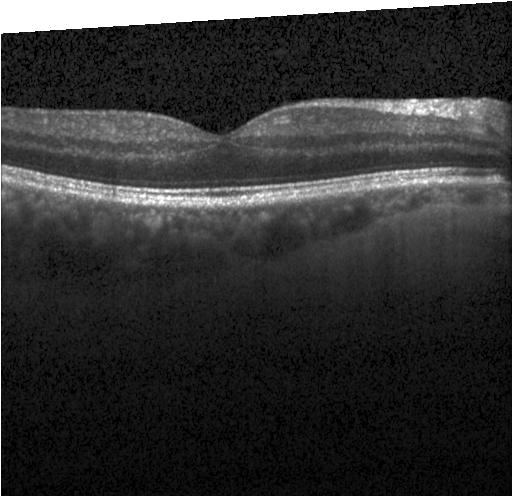

Instrument: Heidelberg Spectralis · spectral-domain optical coherence tomography · retinal OCT B-scan — Diagnosis: no evidence of CNV, DME, or drusen.